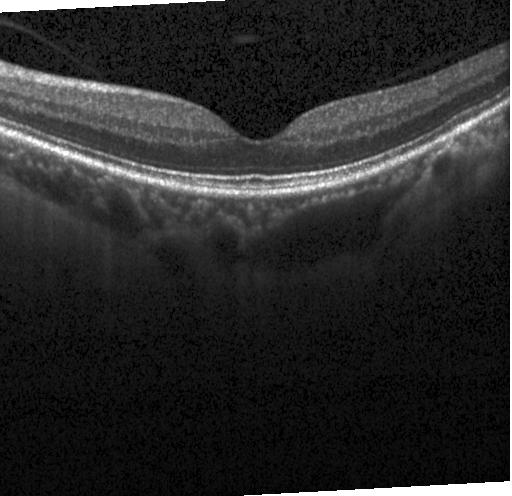
Diagnosis: neither choroidal neovascularization, diabetic macular edema, nor drusen.